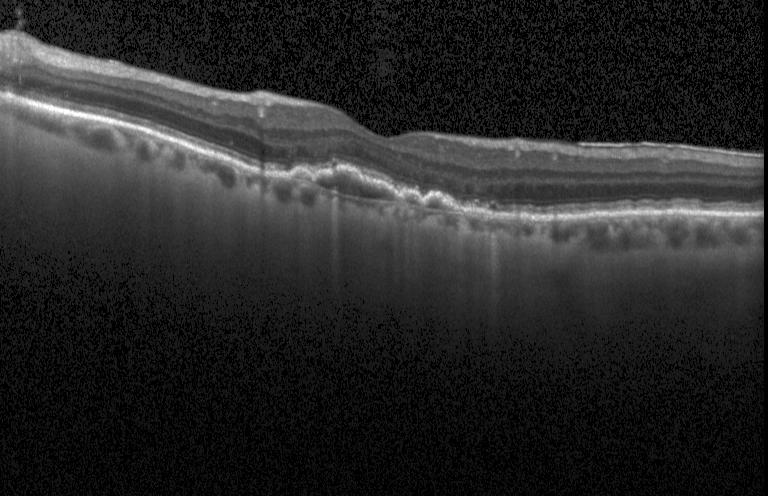 Fovea-centered; retinal OCT B-scan; SD-OCT; instrument: Heidelberg Spectralis.
Choroidal neovascularization (CNV).